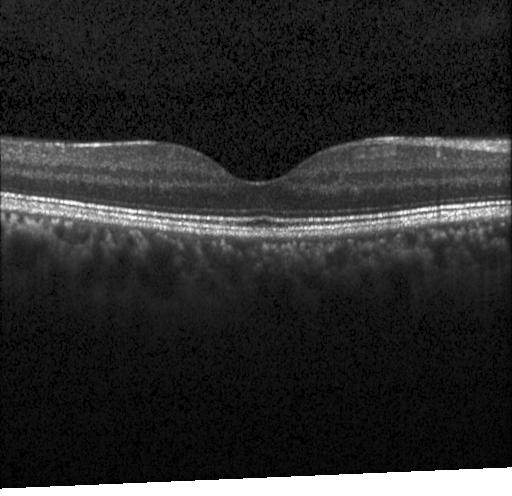 Dx: no evidence of choroidal neovascularization, diabetic macular edema, or drusen.